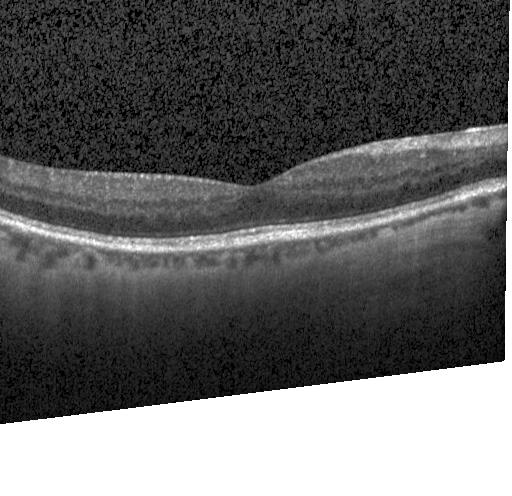 Spectral-domain optical coherence tomography. Optical coherence tomography scan — No evidence of choroidal neovascularization, diabetic macular edema, or drusen.